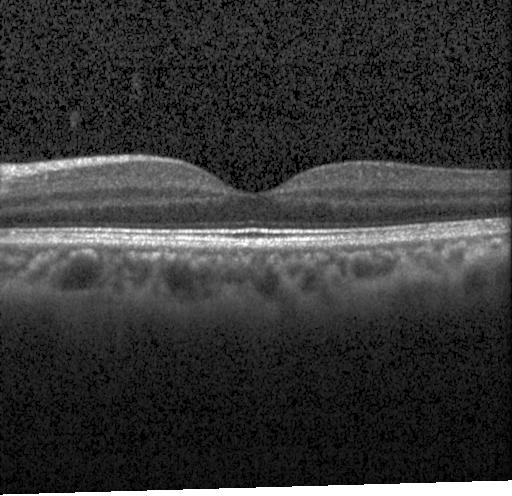
Optical coherence tomography scan, fovea-centered, spectral-domain optical coherence tomography. Impression: no CNV, DME, or drusen.